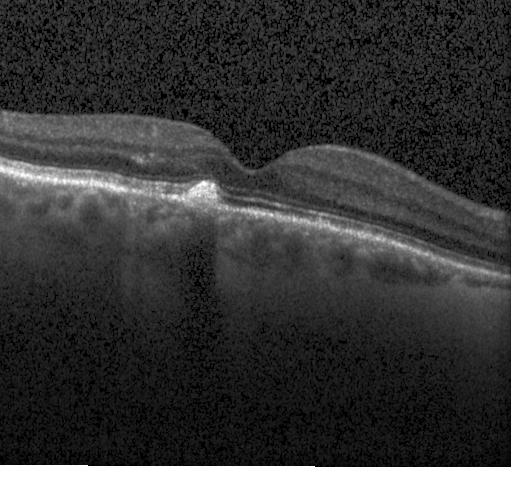 Finding: multiple drusen.